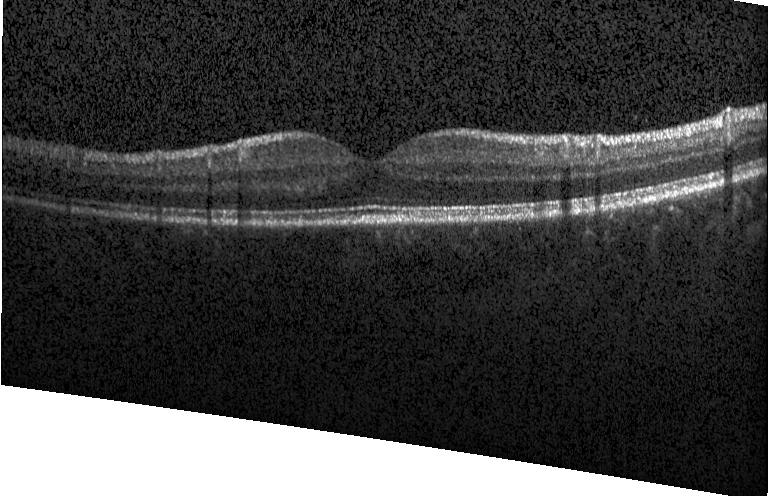 OCT scan showing no choroidal neovascularization, diabetic macular edema, or drusen.